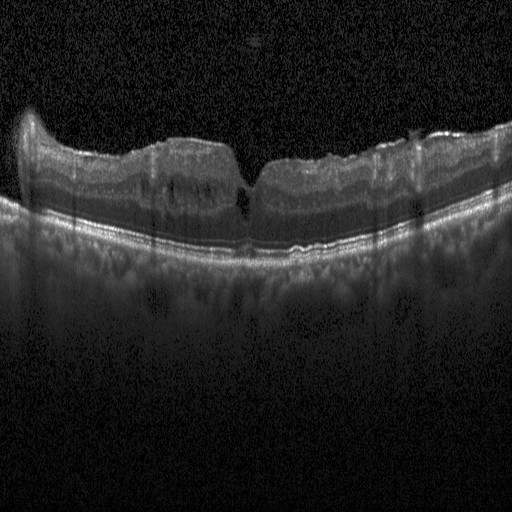
OCT line scan. Fovea-centered — This B-scan demonstrates DME.